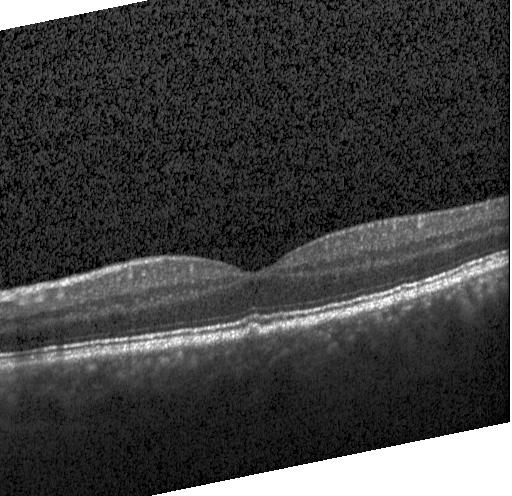
Spectral-domain OCT, OCT B-scan — Impression: multiple drusen.